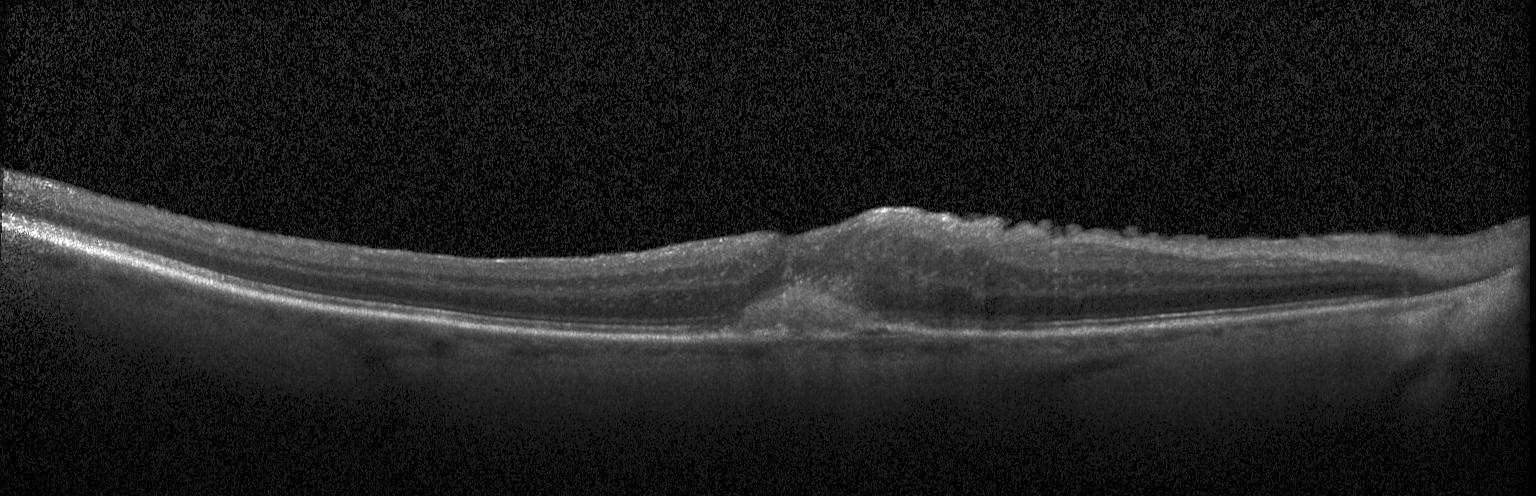
OCT line scan; fovea-centered; spectral-domain OCT. Impression: choroidal neovascularization.